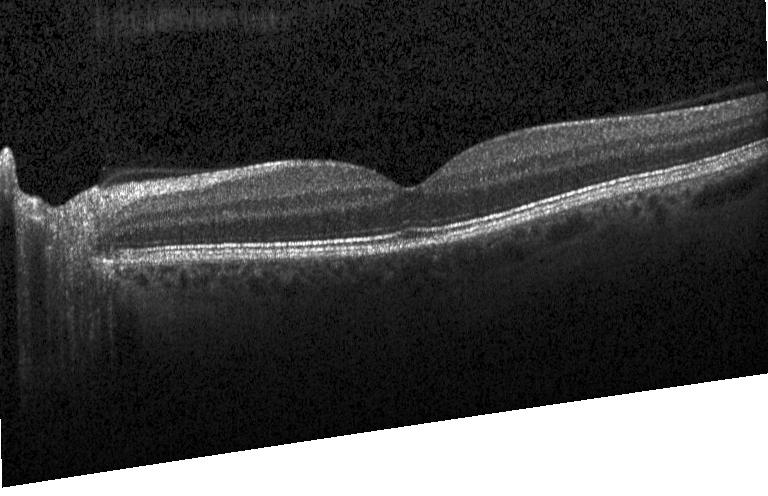 Retinal OCT cross-section showing no CNV, no DME, and no drusen.